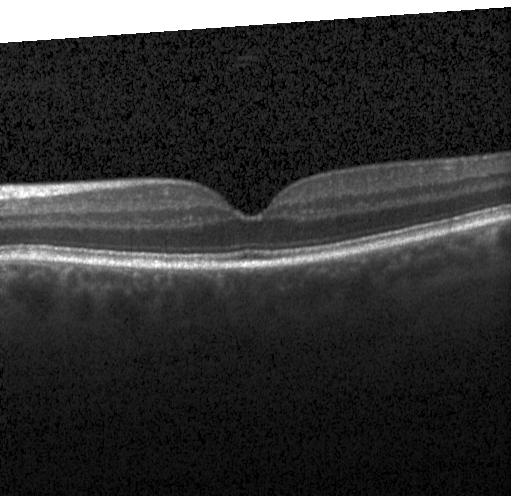 Assessment: no choroidal neovascularization, diabetic macular edema, or drusen.